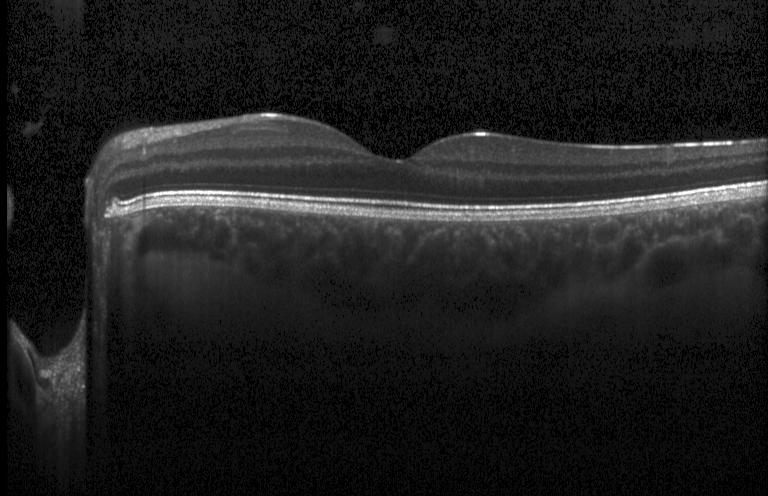 Finding: no choroidal neovascularization, diabetic macular edema, or drusen.